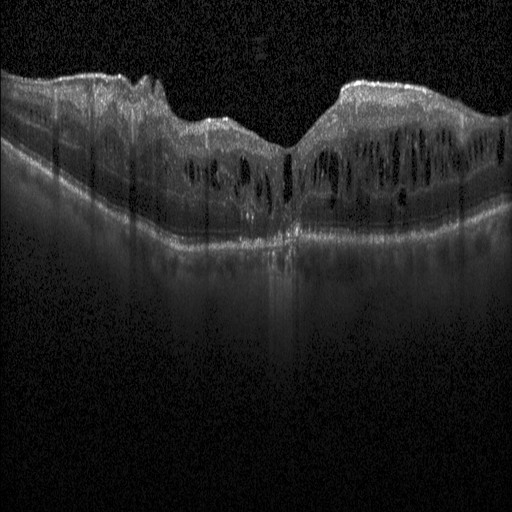
Diabetic macular edema.